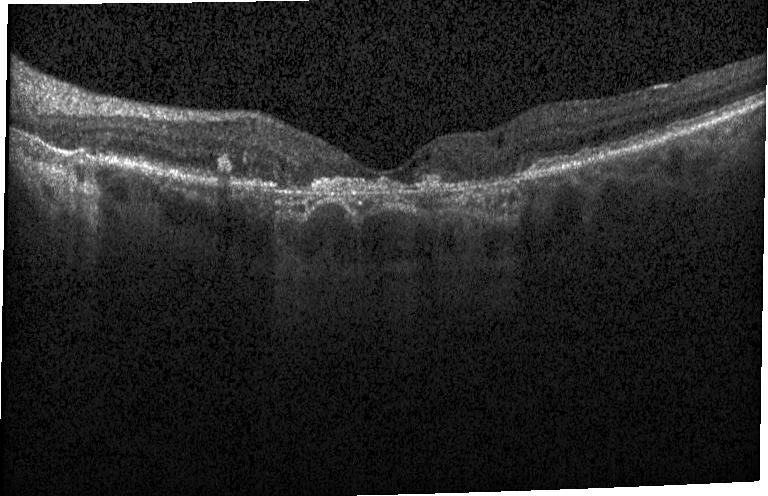

Through the macula · OCT B-scan · spectral-domain OCT · Heidelberg Spectralis
Impression: a choroidal neovascular membrane.